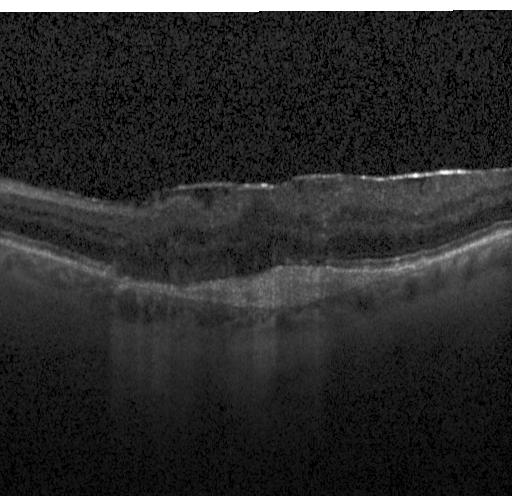 Retinal OCT B-scan.
This B-scan demonstrates a choroidal neovascular membrane.